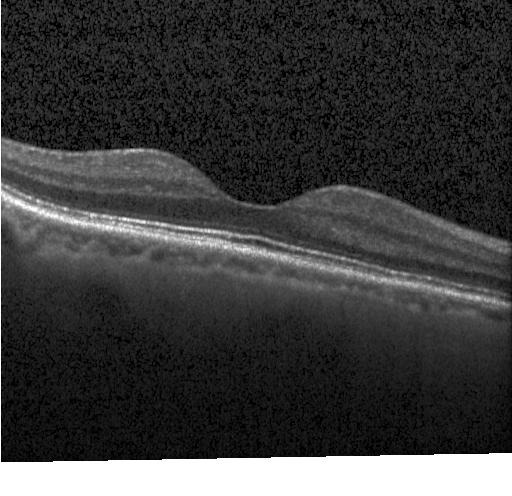

Acquired on a Heidelberg Spectralis; spectral-domain optical coherence tomography; centered on the fovea; optical coherence tomography scan
Diagnosis: no CNV, no DME, and no drusen.